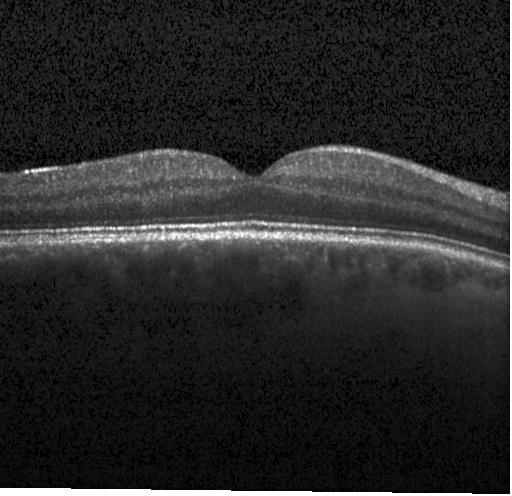 OCT B-scan; Heidelberg Spectralis OCT system — Diagnosis: no choroidal neovascularization, no diabetic macular edema, and no drusen.